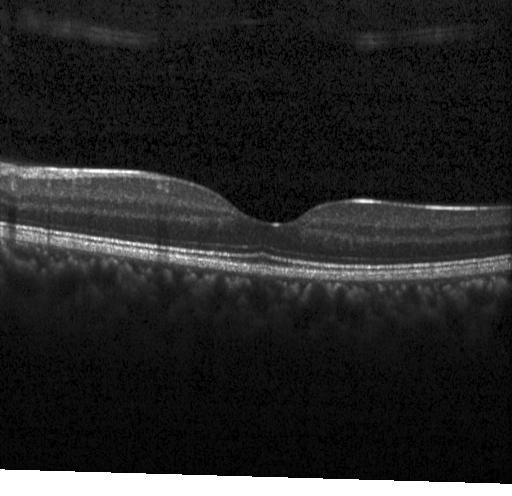

Retinal OCT B-scan. OCT finding: neither choroidal neovascularization, diabetic macular edema, nor drusen.